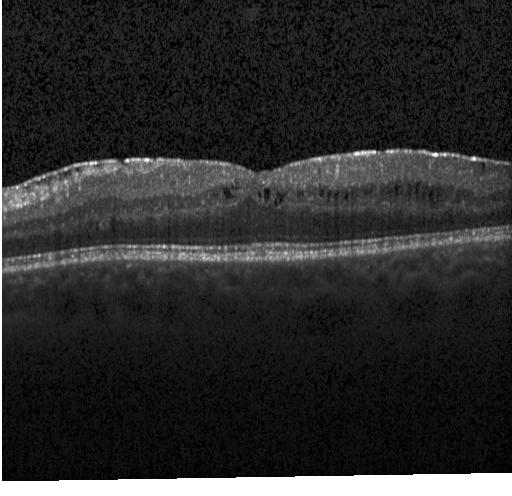 OCT finding: diabetic macular edema (DME).